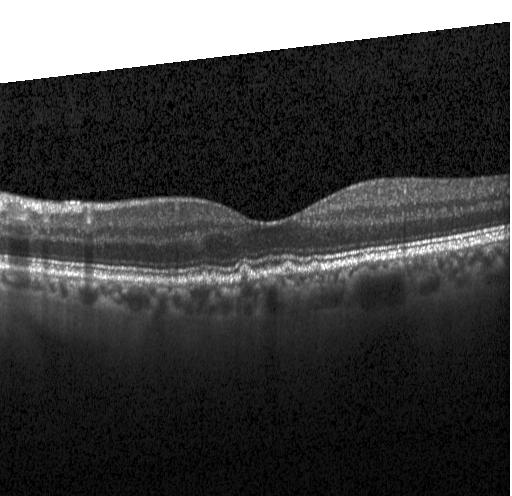

Optical coherence tomography scan. Finding: multiple drusen.